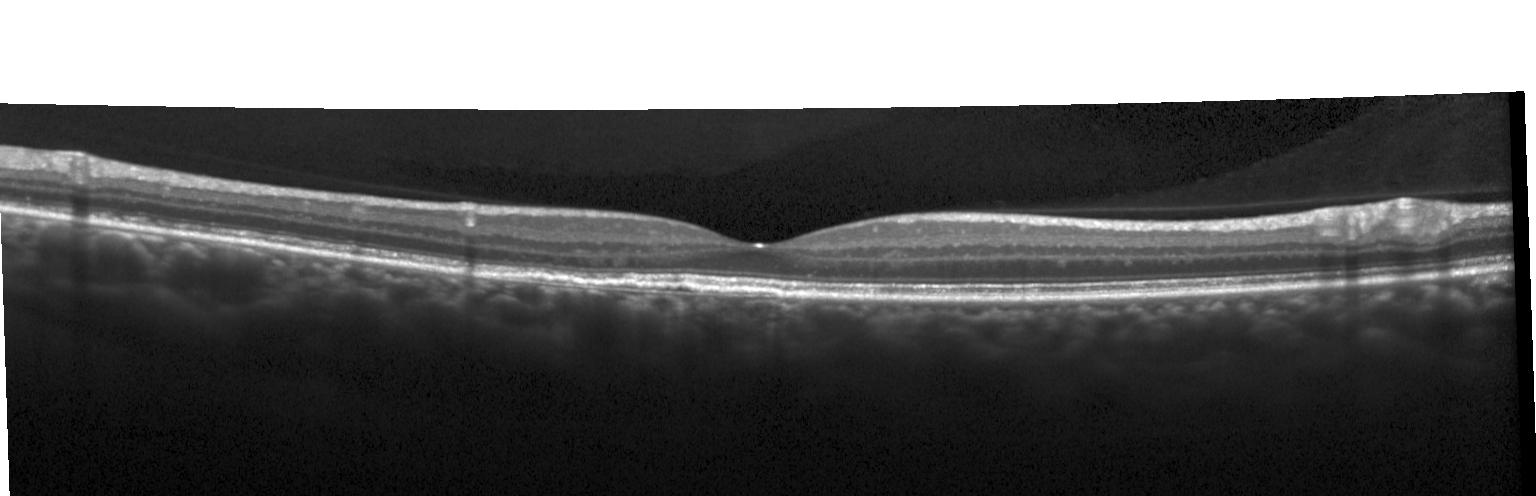 No CNV, DME, or drusen.